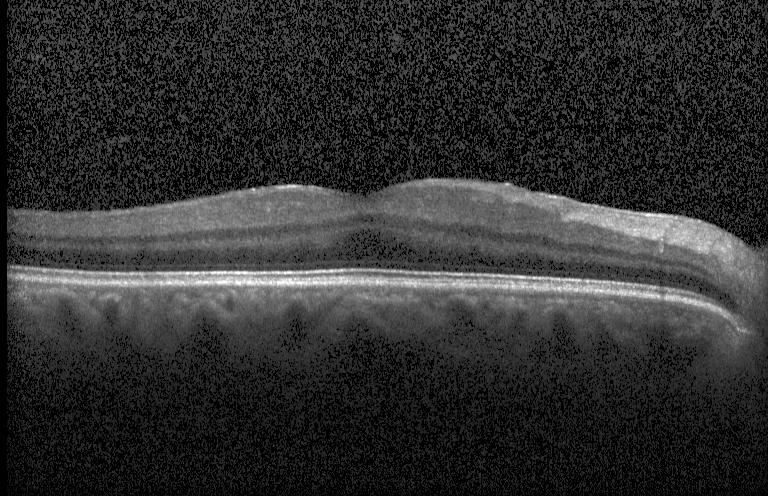 Macular scan. Spectral-domain optical coherence tomography. Heidelberg Spectralis OCT system. Retinal OCT cross-section. OCT finding: neither choroidal neovascularization, diabetic macular edema, nor drusen.